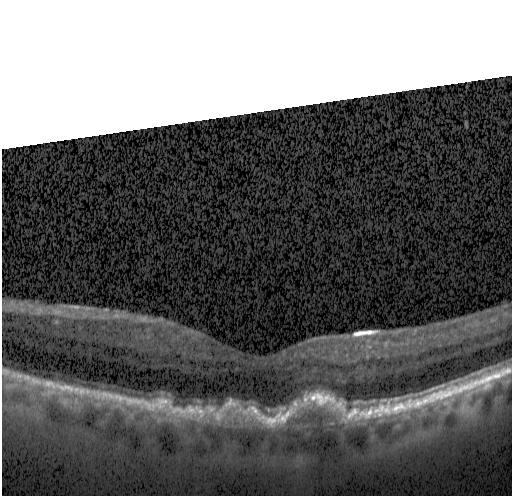 Instrument: Heidelberg Spectralis; spectral-domain OCT; retinal OCT B-scan — Impression: multiple drusen.